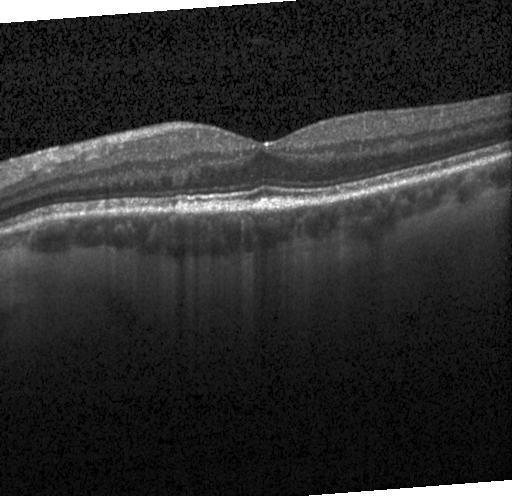
OCT line scan.
No choroidal neovascularization, no diabetic macular edema, and no drusen.